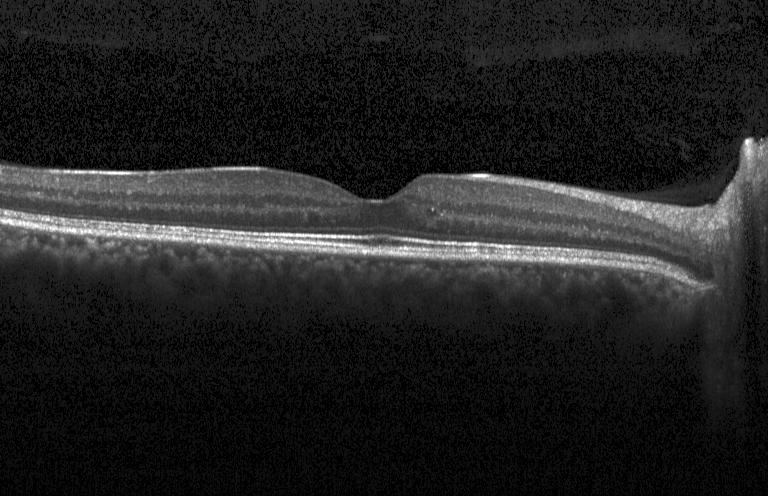
This B-scan demonstrates no choroidal neovascularization, no diabetic macular edema, and no drusen.